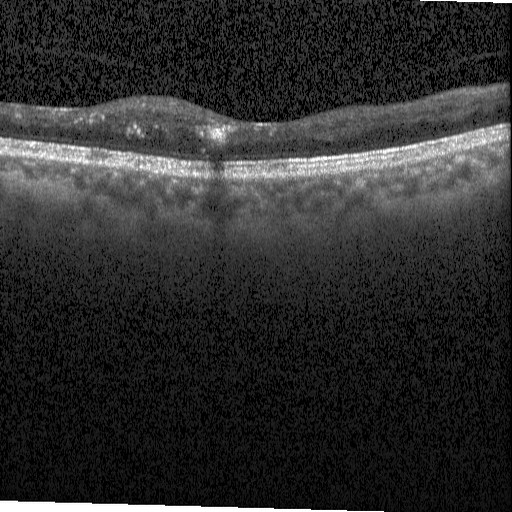 Instrument: Heidelberg Spectralis, retinal OCT B-scan, fovea-centered, SD-OCT.
Assessment: DME.